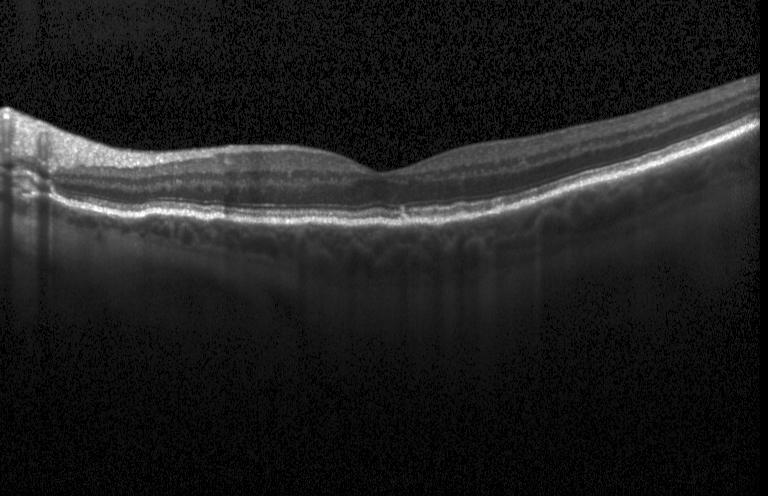 Optical coherence tomography scan; spectral-domain OCT; through the macula. This B-scan demonstrates multiple drusen.